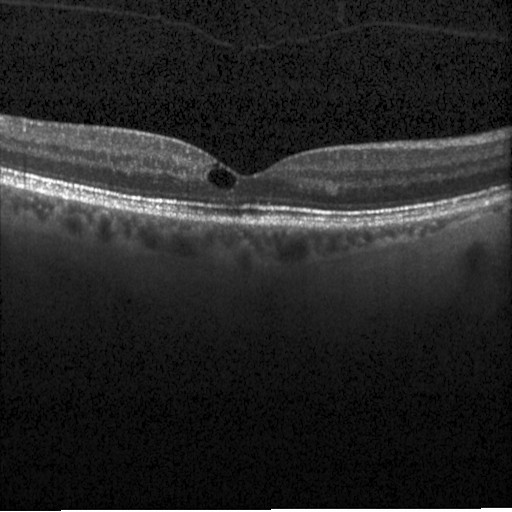
Instrument: Heidelberg Spectralis; retinal OCT cross-section; spectral-domain OCT — Diabetic macular edema (DME).